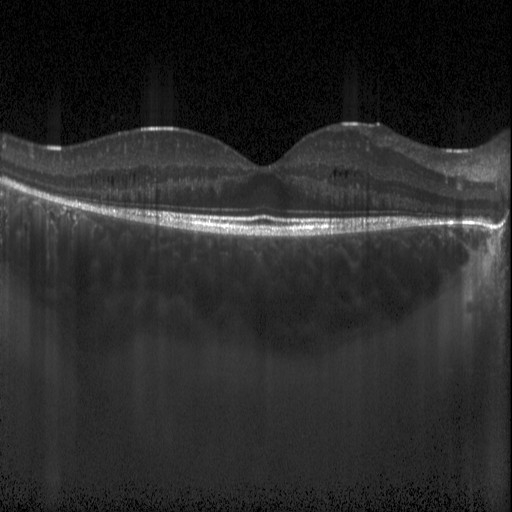

Spectral-domain OCT · OCT line scan — Assessment: diabetic macular edema (DME).